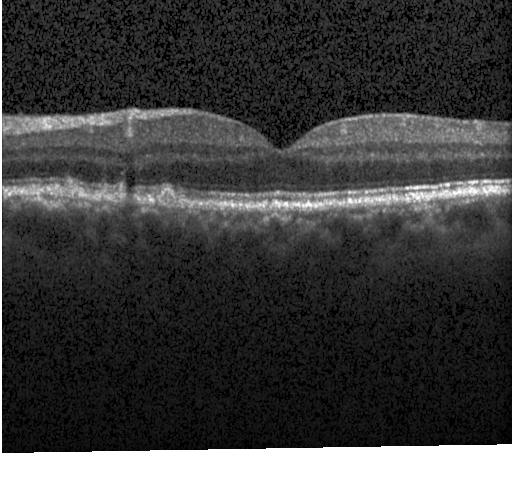
Horizontal scan through the fovea. OCT B-scan. SD-OCT — Impression: multiple drusen.